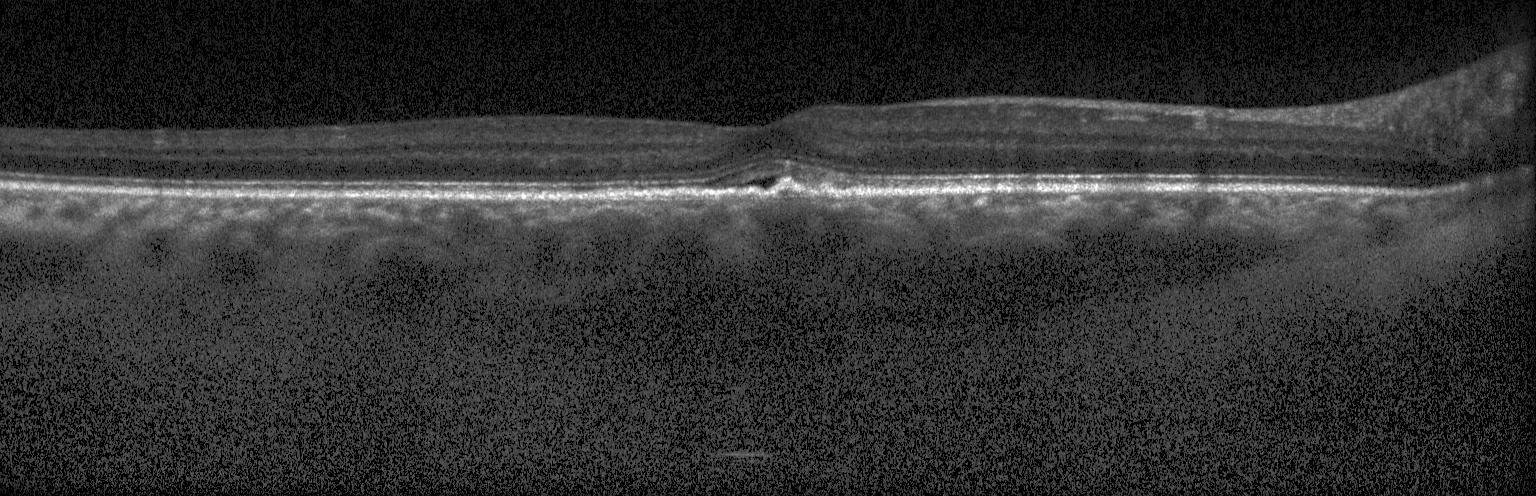 Heidelberg Spectralis OCT system. Retinal OCT cross-section
CNV.